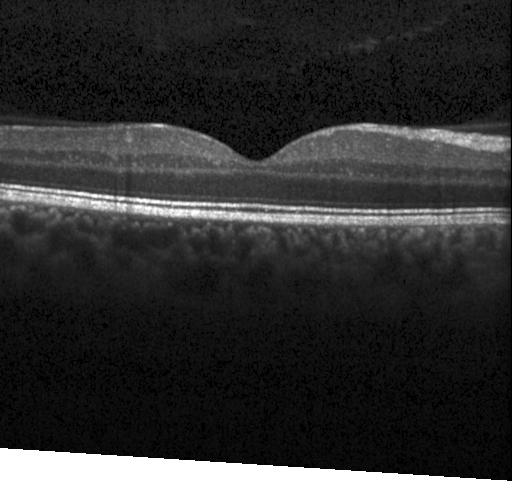
Optical coherence tomography B-scan. Instrument: Heidelberg Spectralis — Neither choroidal neovascularization, diabetic macular edema, nor drusen.